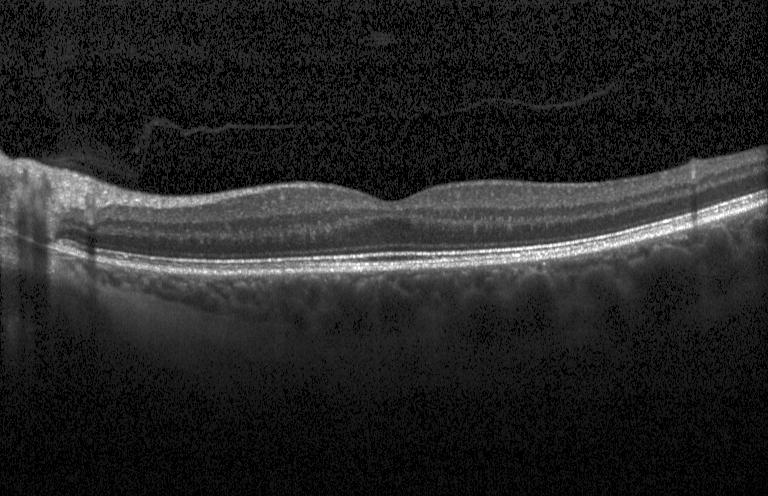
No CNV, no DME, and no drusen.